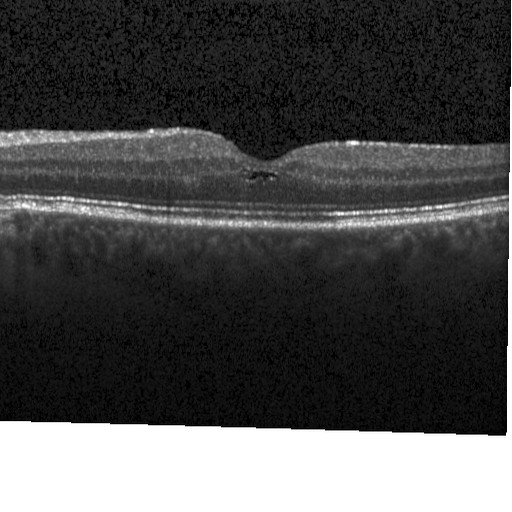

Retinal OCT B-scan. This B-scan demonstrates diabetic macular edema (DME).